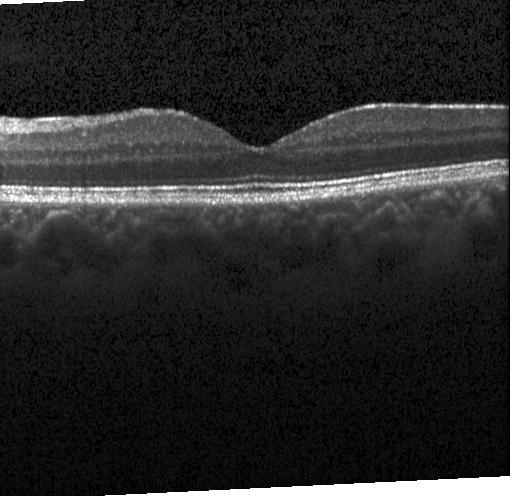

OCT B-scan. Impression: no CNV, no DME, and no drusen.